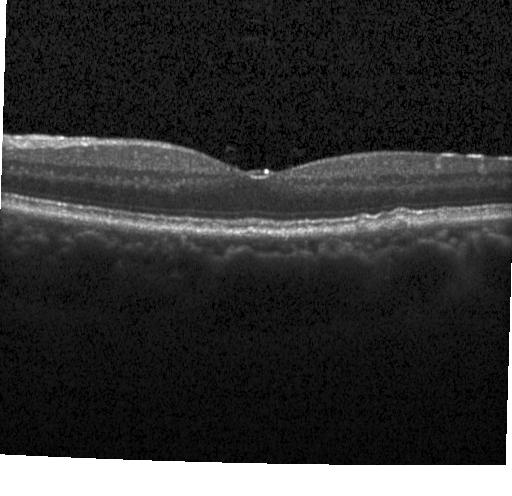 Diagnosis: multiple drusen.